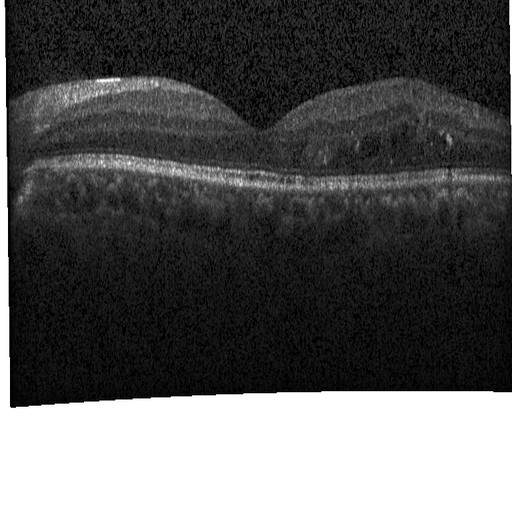 Heidelberg Spectralis OCT system. Optical coherence tomography scan. Dx: diabetic macular edema.